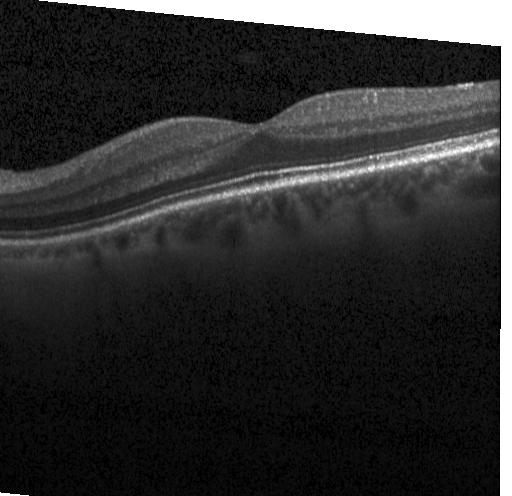

Spectral-domain optical coherence tomography; Heidelberg Spectralis OCT system; retinal OCT cross-section; through the macula. Dx: no evidence of choroidal neovascularization, diabetic macular edema, or drusen.